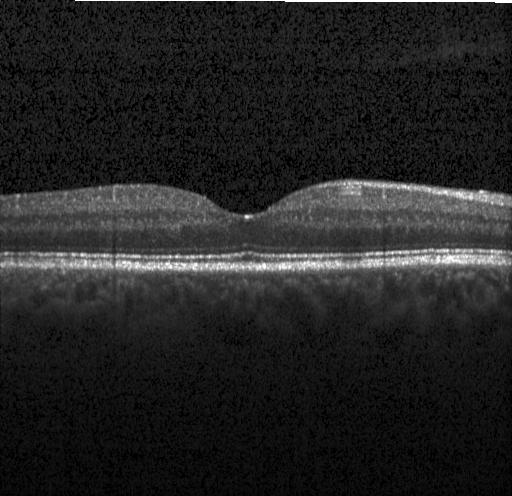

Finding: no choroidal neovascularization, no diabetic macular edema, and no drusen.